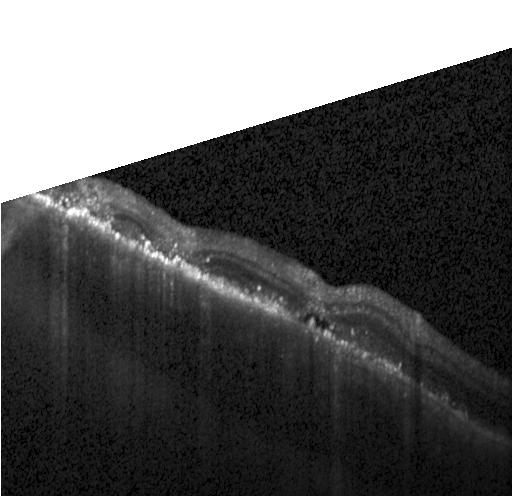

Centered on the fovea, spectral-domain OCT, retinal OCT cross-section — Finding: choroidal neovascularization.